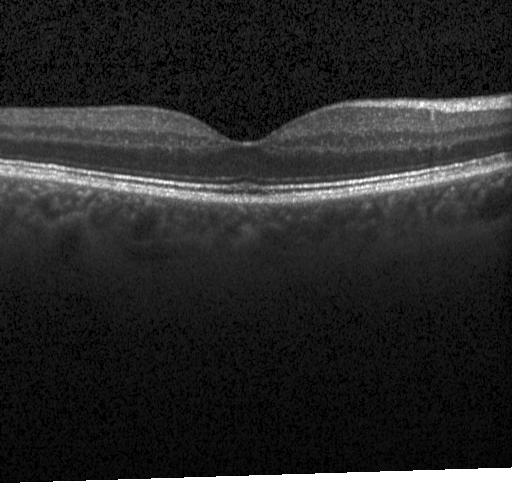 Heidelberg Spectralis, retinal OCT cross-section, spectral-domain OCT
Finding: neither CNV, DME, nor drusen.